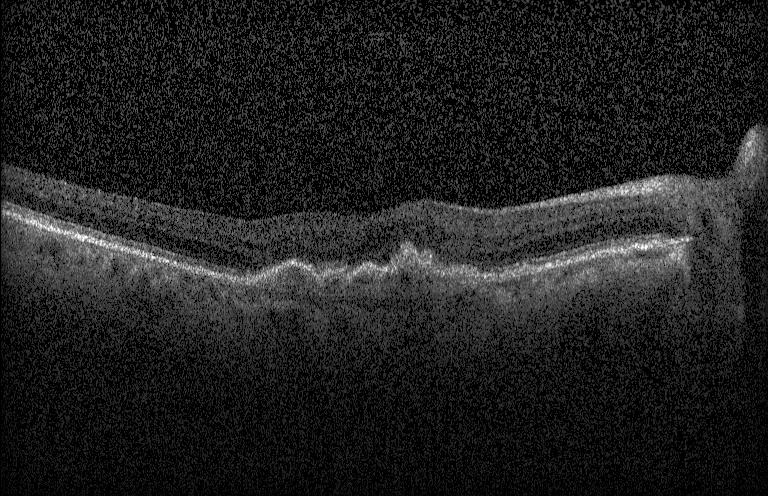 Spectral-domain OCT; OCT line scan; through the macula. A choroidal neovascular membrane.